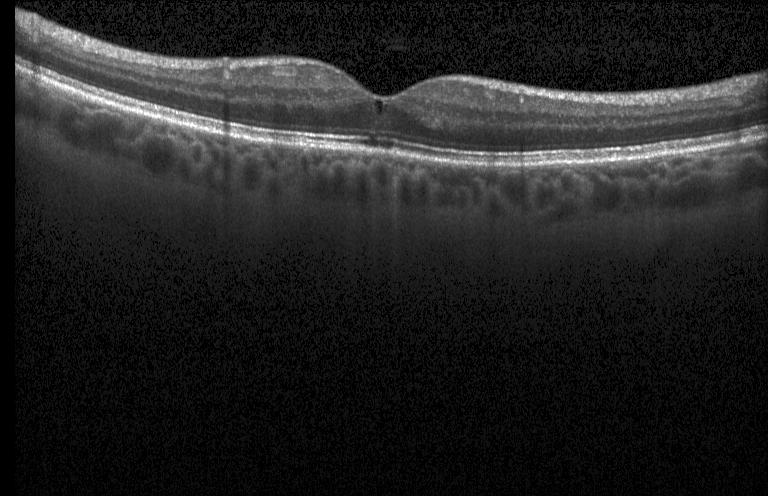

Assessment: DME.